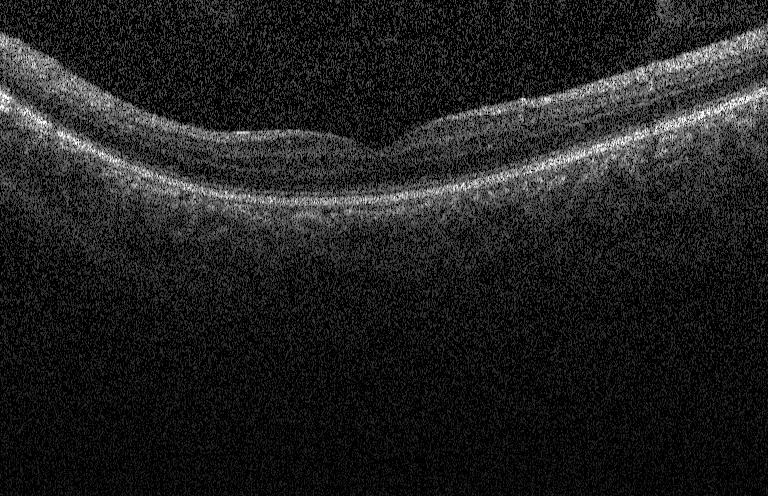 Spectral-domain OCT. Fovea-centered. Retinal OCT cross-section. Impression: no choroidal neovascularization, diabetic macular edema, or drusen.